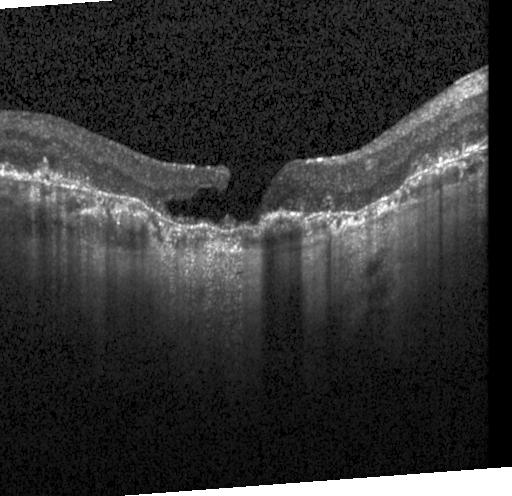

Acquired on a Heidelberg Spectralis; OCT line scan; SD-OCT; macular scan.
Diagnosis: CNV.